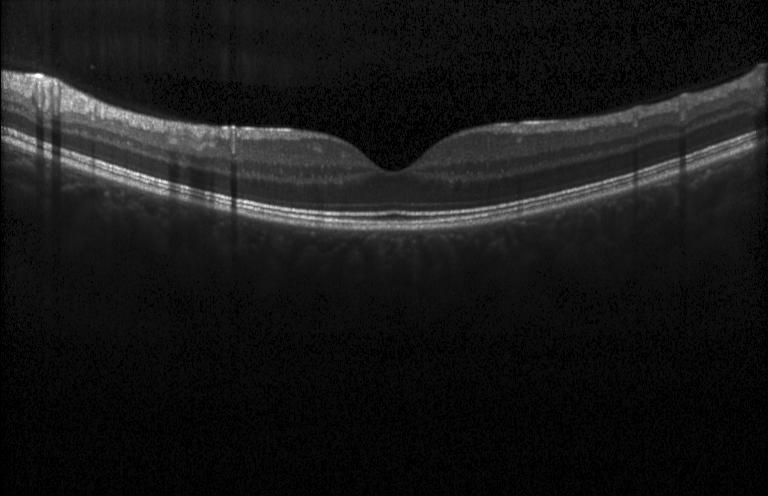

Retinal OCT cross-section, through the macula — Assessment: no CNV, DME, or drusen.